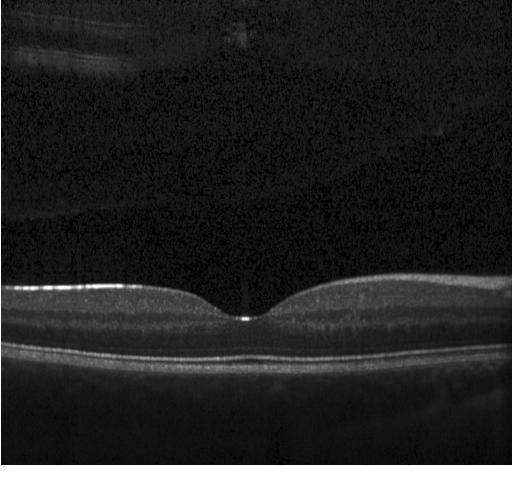

Diagnosis: no choroidal neovascularization, diabetic macular edema, or drusen.